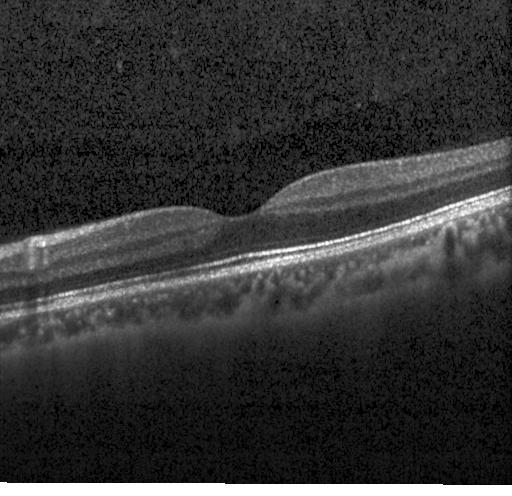

Finding: neither choroidal neovascularization, diabetic macular edema, nor drusen.